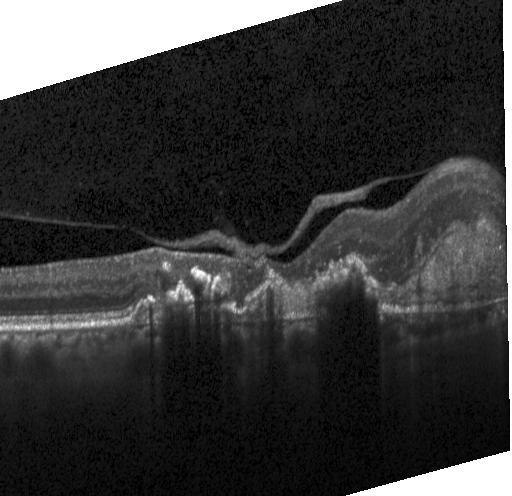 Heidelberg Spectralis · spectral-domain optical coherence tomography · OCT line scan
Choroidal neovascularization (CNV).